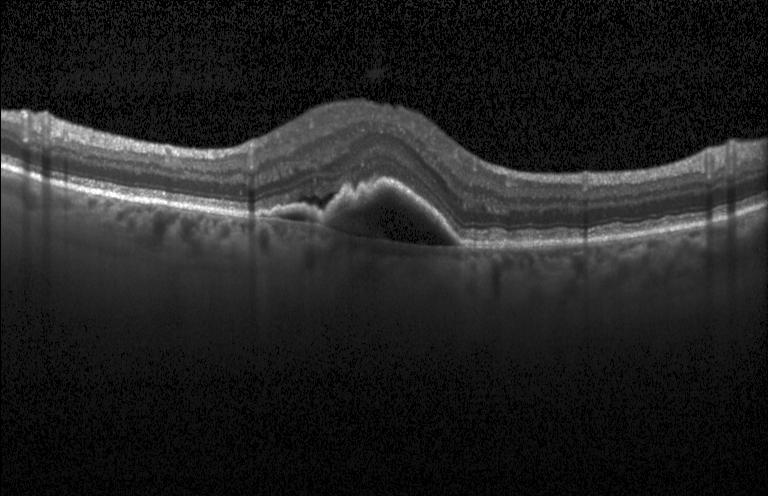
Impression: choroidal neovascularization (CNV).